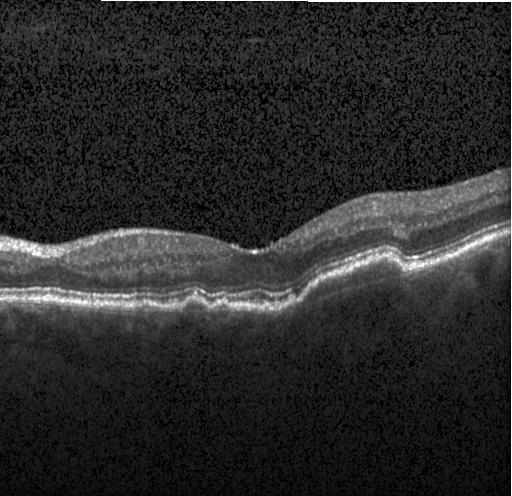

Through the macula, OCT B-scan — Diagnosis: a choroidal neovascular membrane.